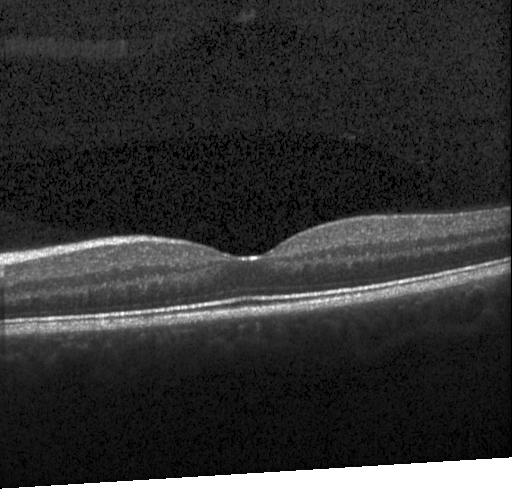
Spectral-domain OCT, Heidelberg Spectralis, macular scan, OCT B-scan. Diagnosis: no choroidal neovascularization, diabetic macular edema, or drusen.